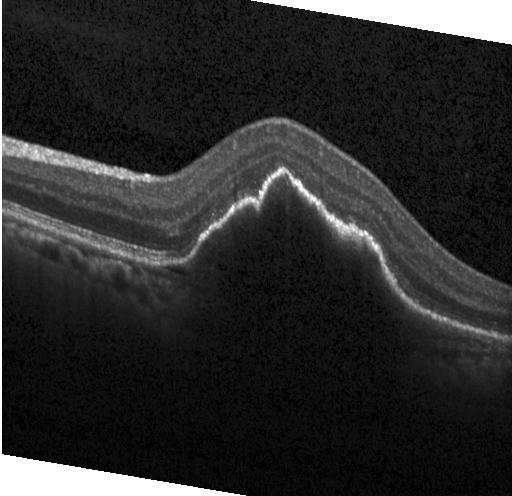 Retinal OCT cross-section. Through the macula. Spectral-domain OCT.
Macular OCT: choroidal neovascularization (CNV).